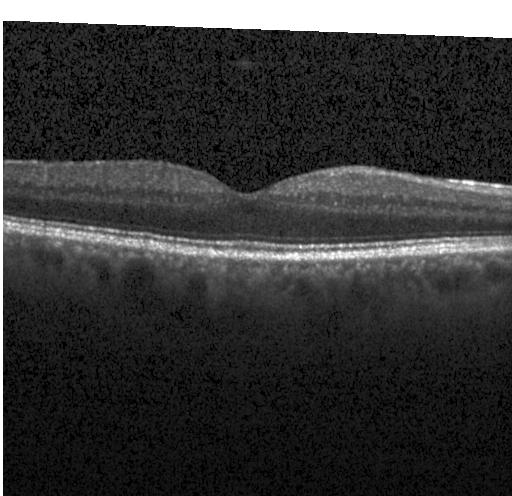
Macular OCT demonstrating no choroidal neovascularization, no diabetic macular edema, and no drusen.